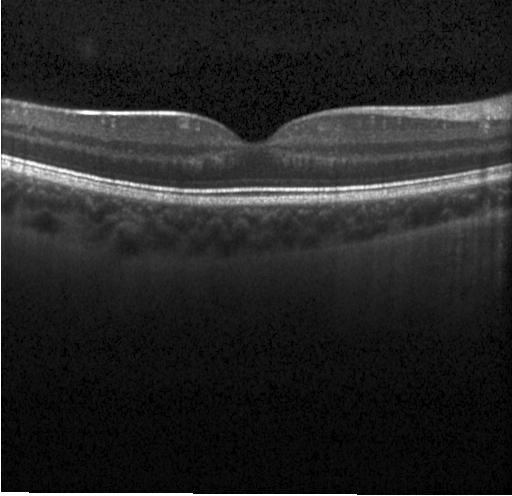 Optical coherence tomography scan — Diagnosis: no CNV, DME, or drusen.